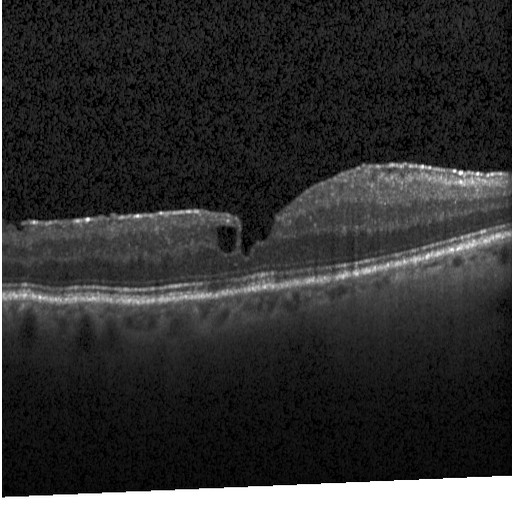
OCT finding: diabetic macular edema (DME).